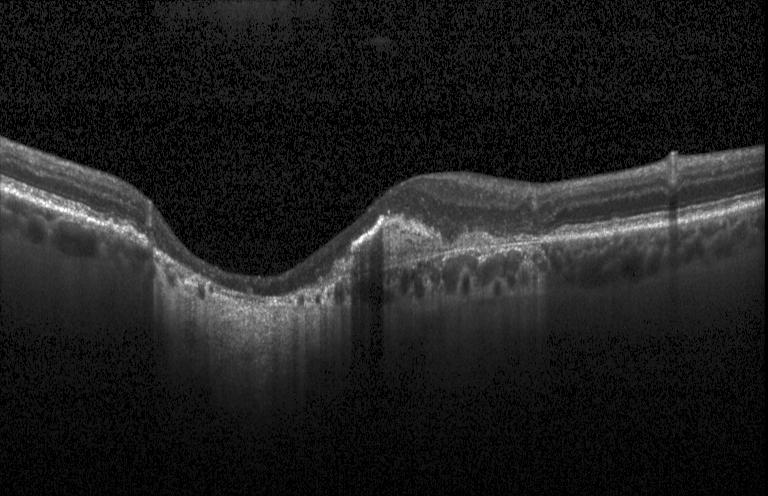

Finding: choroidal neovascularization.